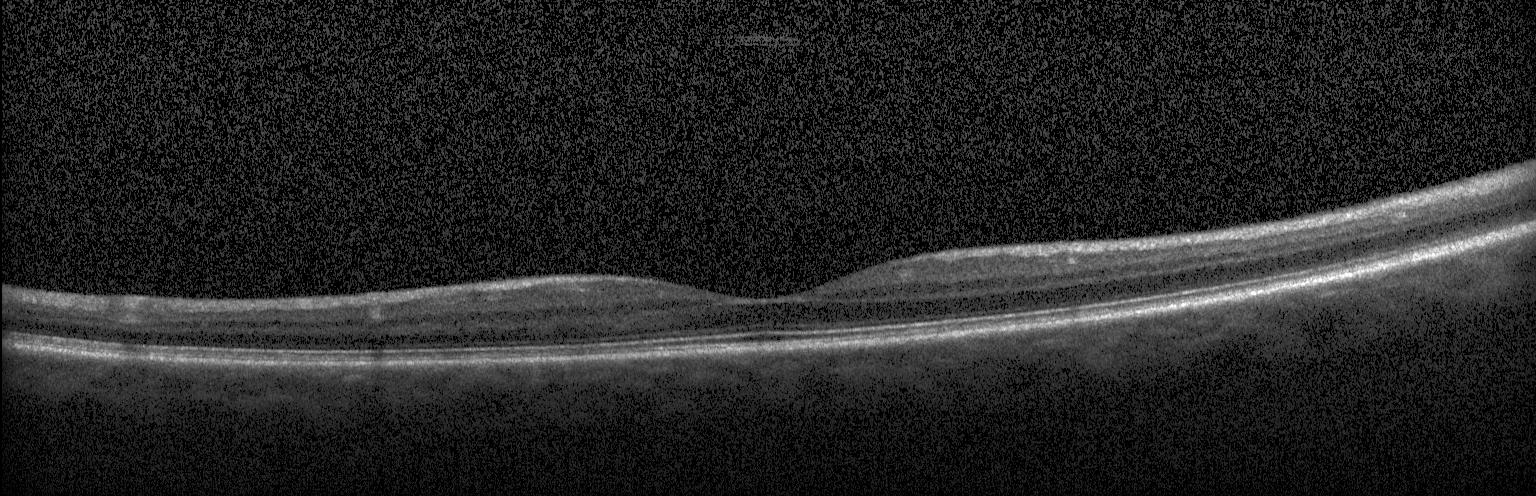

Macular OCT demonstrating no choroidal neovascularization, diabetic macular edema, or drusen.